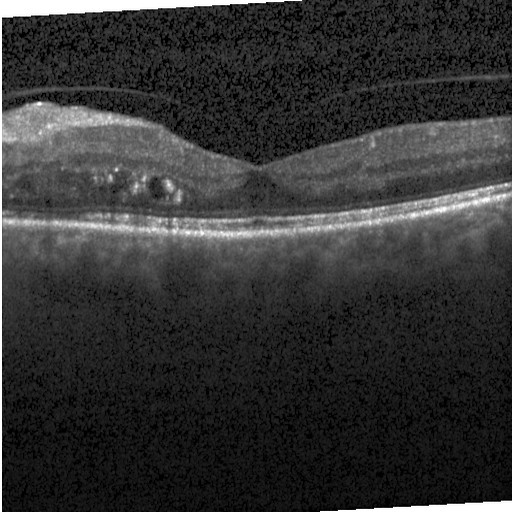 Retinal OCT cross-section showing diabetic macular edema (DME).